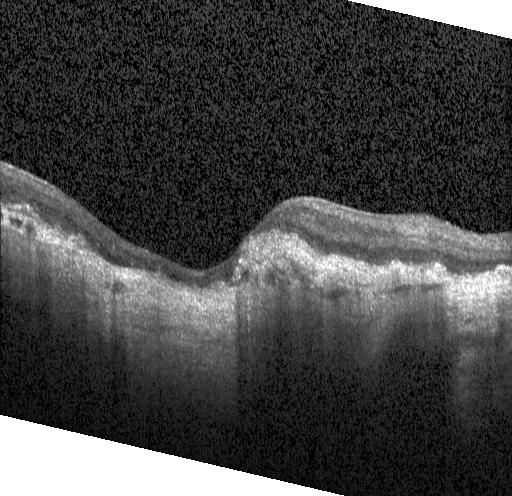
OCT B-scan; Heidelberg Spectralis OCT system
CNV.